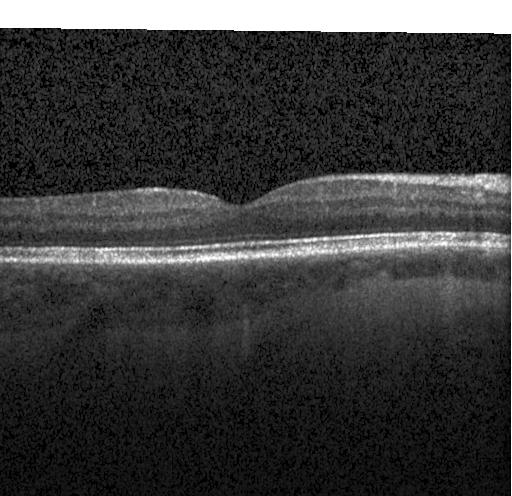
OCT scan showing no evidence of CNV, DME, or drusen.